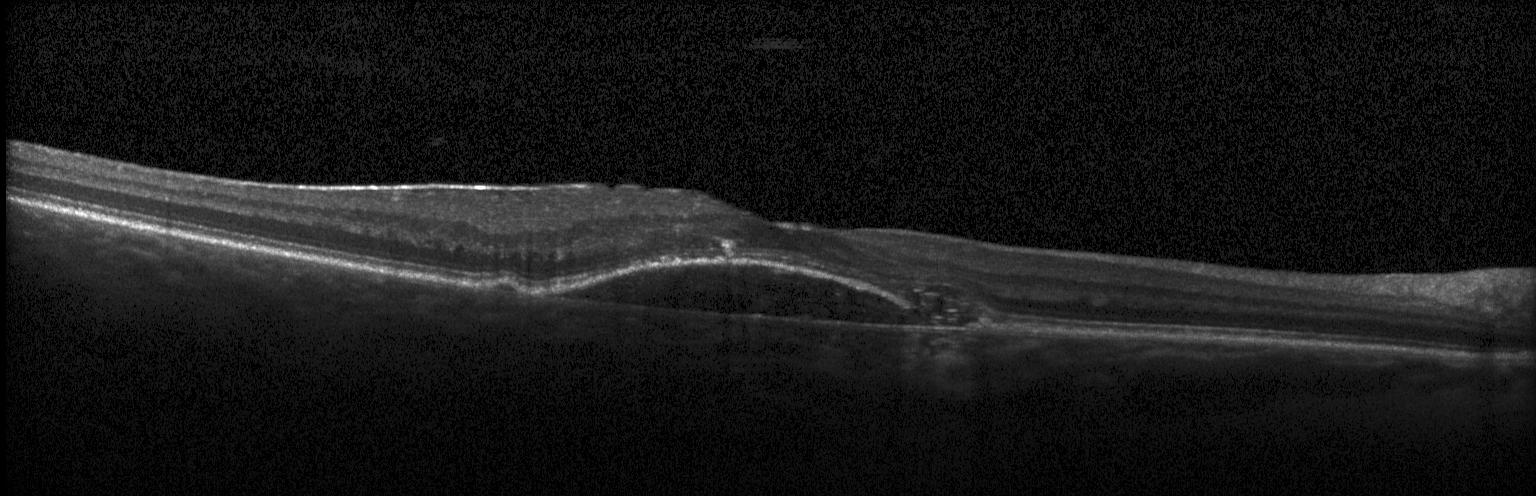

Horizontal scan through the fovea, OCT line scan — Finding: a choroidal neovascular membrane.